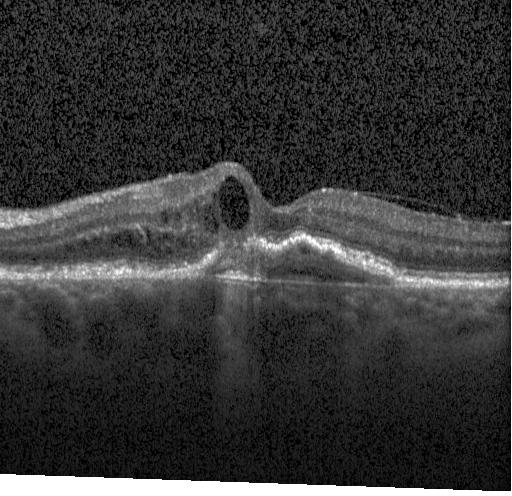
Optical coherence tomography scan
Impression: a choroidal neovascular membrane.